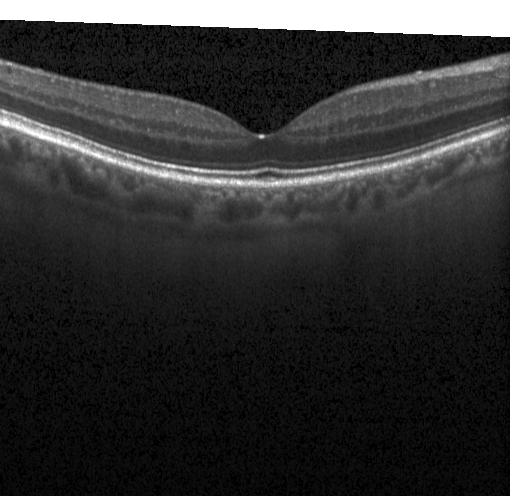

OCT line scan, macular scan
This B-scan demonstrates no evidence of CNV, DME, or drusen.